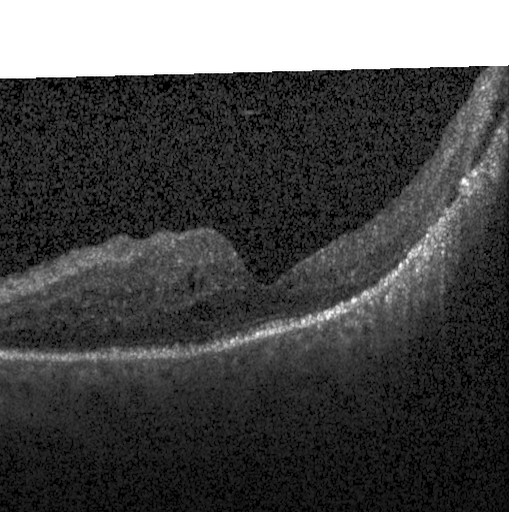
Optical coherence tomography scan
This B-scan demonstrates diabetic macular edema.